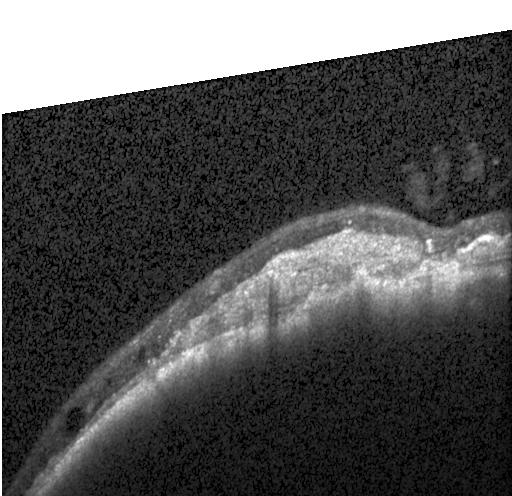
Retinal OCT cross-section showing CNV.